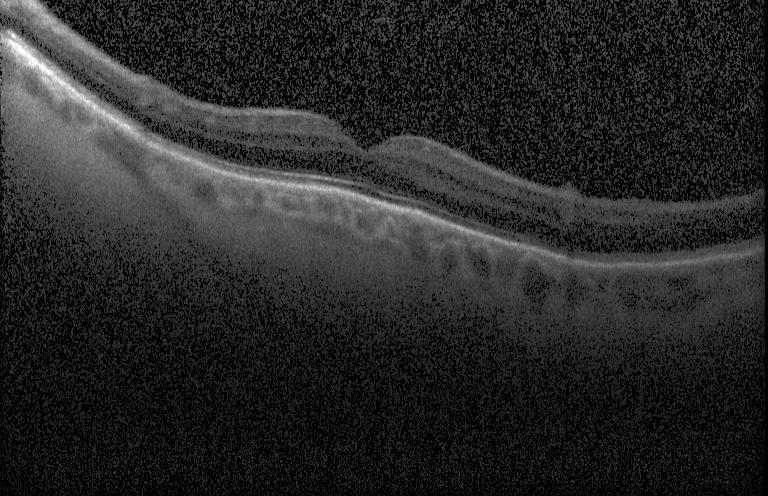
Centered on the fovea · optical coherence tomography scan · Heidelberg Spectralis OCT system · spectral-domain optical coherence tomography — No CNV, DME, or drusen.